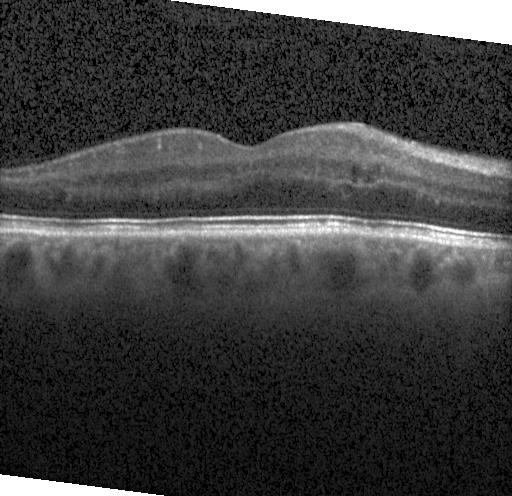 Dx: DME.